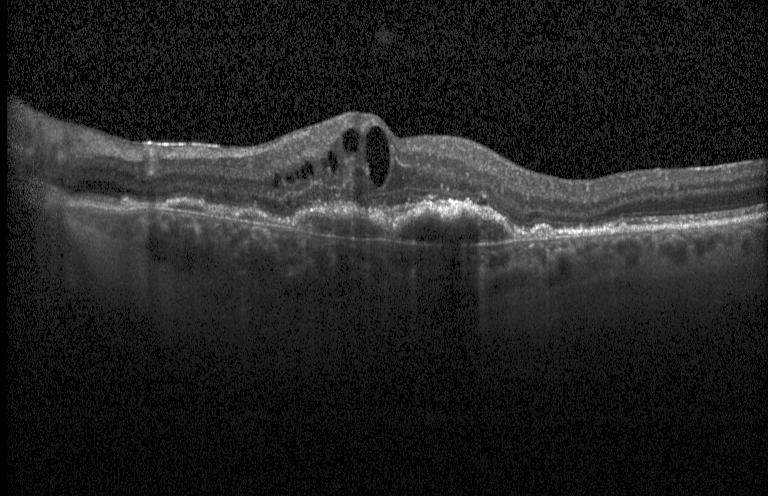 Finding: a choroidal neovascular membrane.